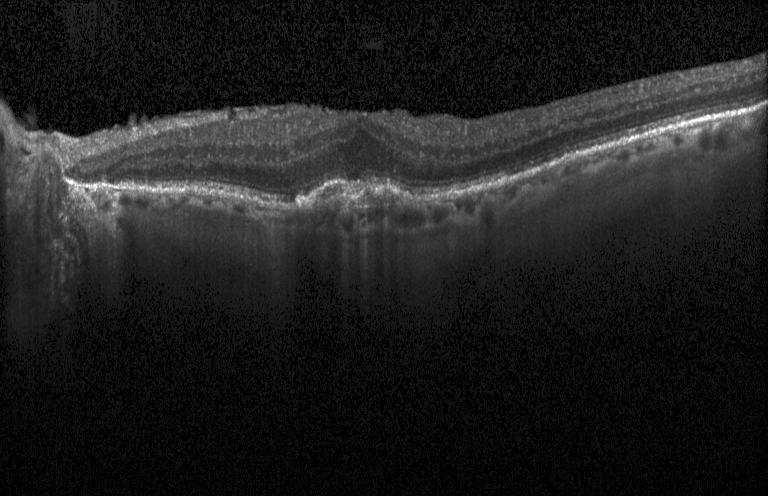

Optical coherence tomography B-scan — Diagnosis: a choroidal neovascular membrane.